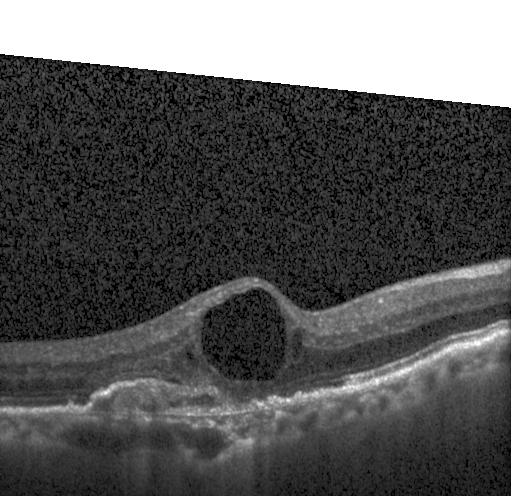
SD-OCT; acquired on a Heidelberg Spectralis; centered on the fovea; OCT line scan — This B-scan demonstrates a choroidal neovascular membrane.